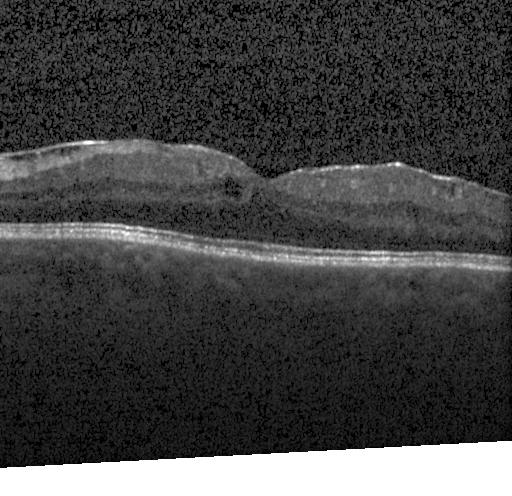 OCT B-scan.
Macular OCT: diabetic macular edema (DME).